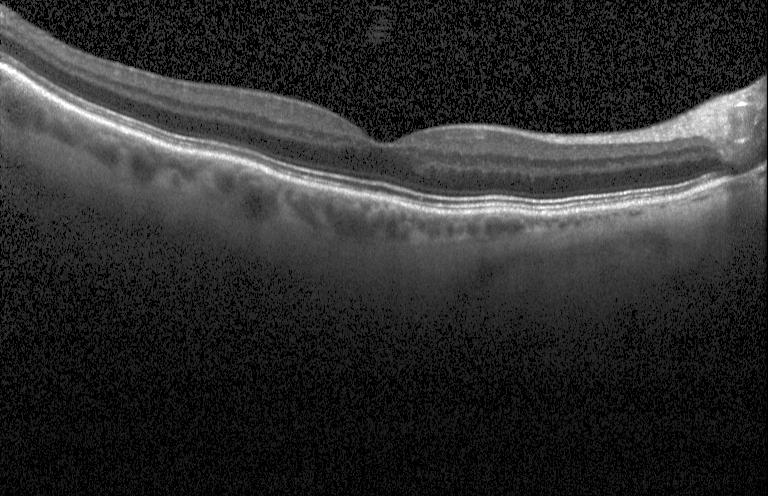
Retinal OCT cross-section
Diagnosis: neither choroidal neovascularization, diabetic macular edema, nor drusen.